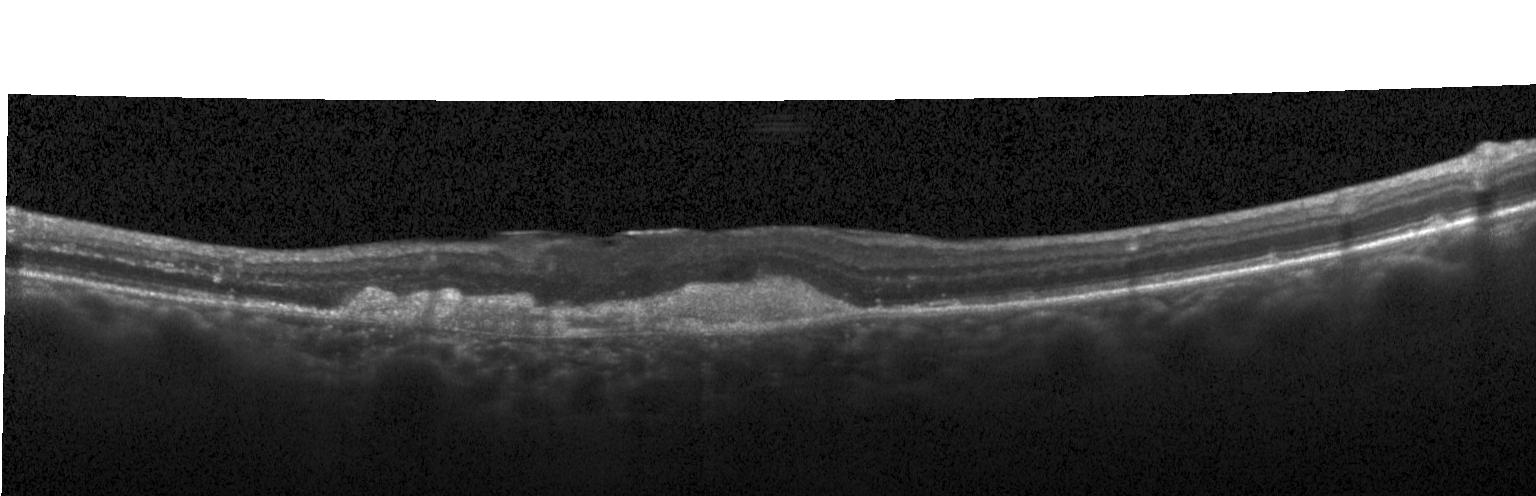 Retinal OCT B-scan
The scan shows choroidal neovascularization (CNV).